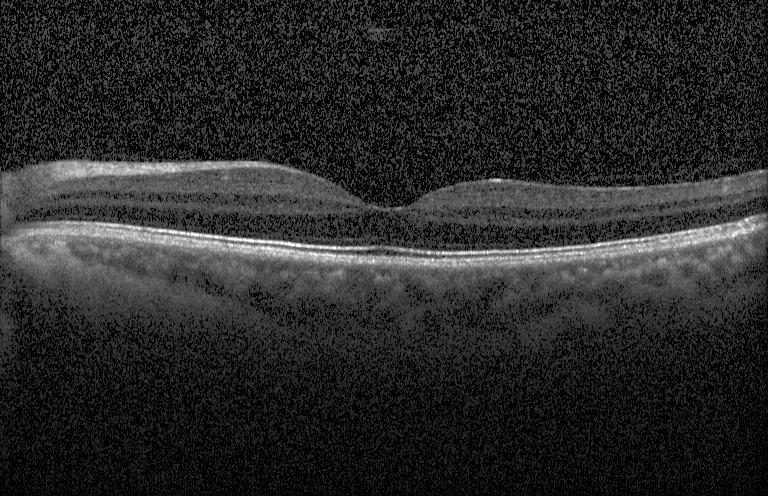

Dx: no CNV, DME, or drusen.